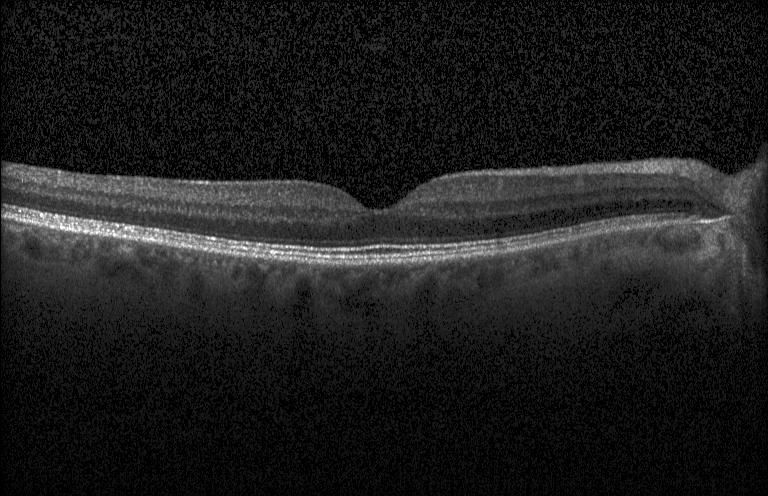 The scan shows no evidence of choroidal neovascularization, diabetic macular edema, or drusen.